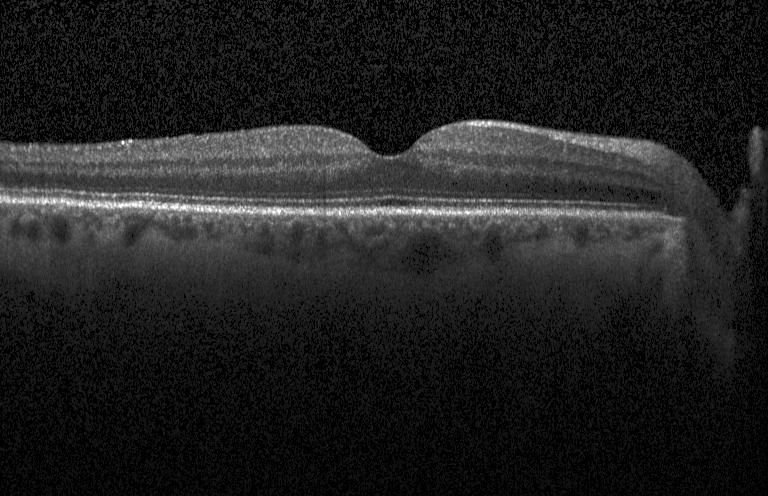

OCT line scan
OCT finding: neither choroidal neovascularization, diabetic macular edema, nor drusen.